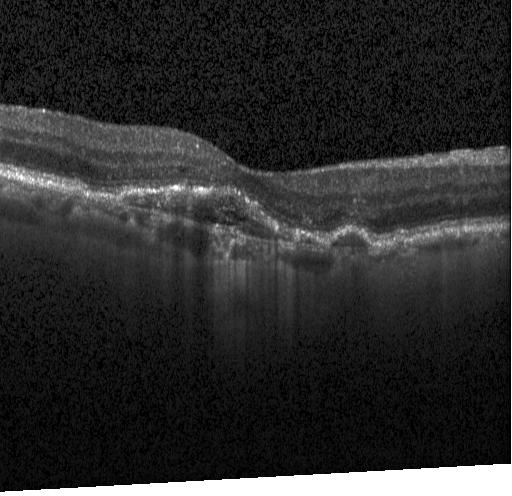
OCT line scan — Finding: CNV.